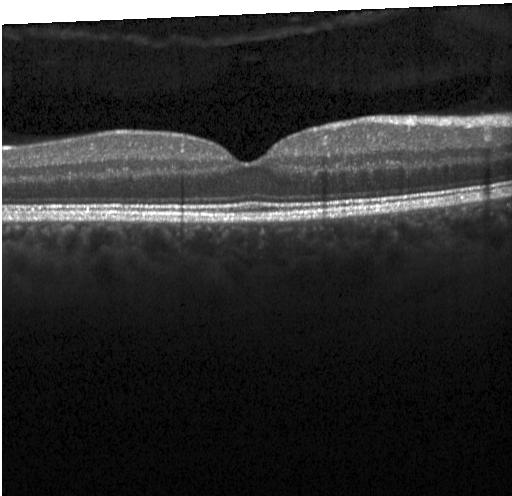 Instrument: Heidelberg Spectralis; spectral-domain optical coherence tomography; optical coherence tomography B-scan; centered on the fovea — Neither choroidal neovascularization, diabetic macular edema, nor drusen.